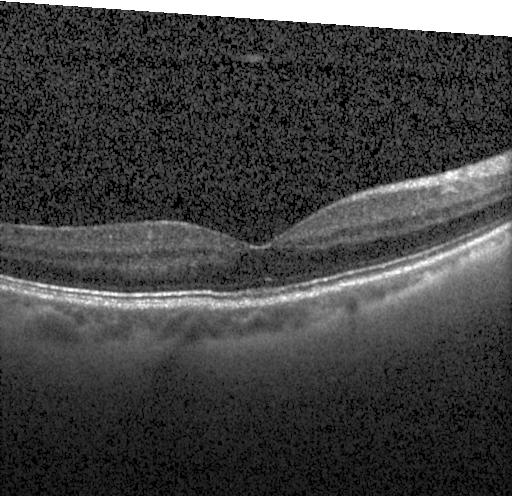

Centered on the fovea · spectral-domain optical coherence tomography · optical coherence tomography scan. Diagnosis: no CNV, no DME, and no drusen.